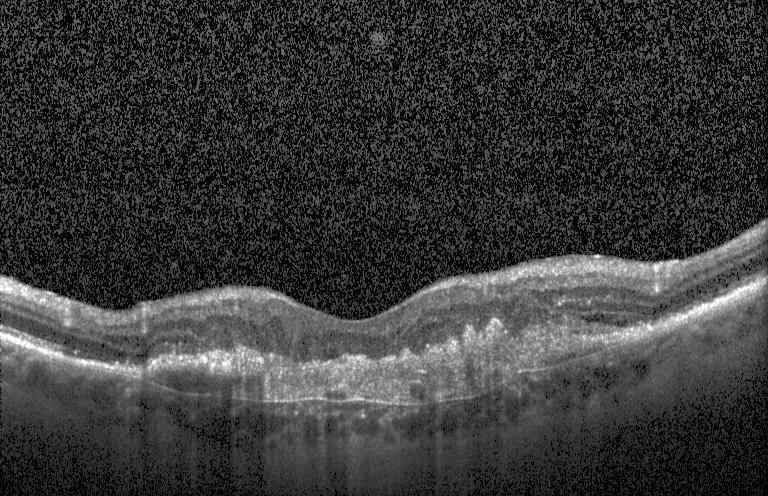 Finding: choroidal neovascularization (CNV).